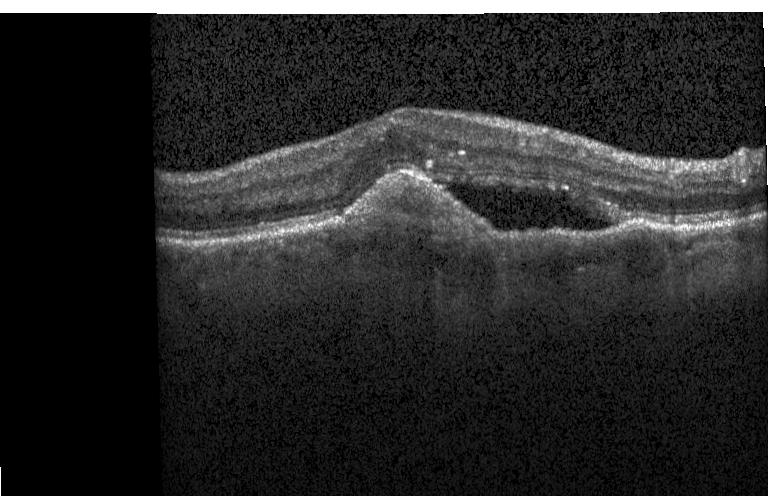 Optical coherence tomography B-scan · horizontal scan through the fovea — Finding: CNV.